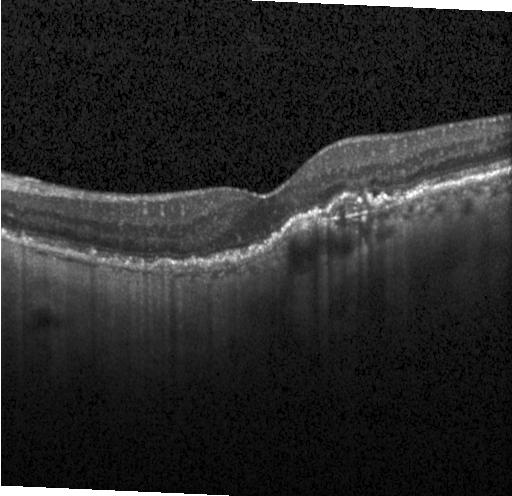

Horizontal scan through the fovea, retinal OCT B-scan. OCT finding: CNV.